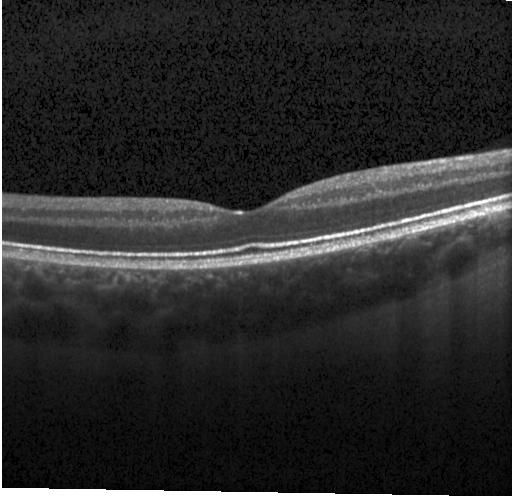

Impression: no choroidal neovascularization, no diabetic macular edema, and no drusen.